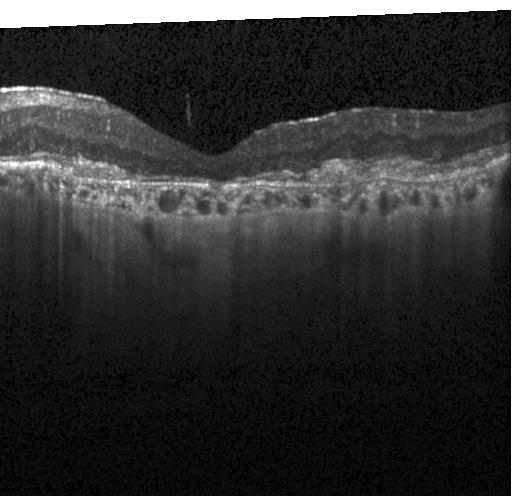
Dx: a choroidal neovascular membrane.